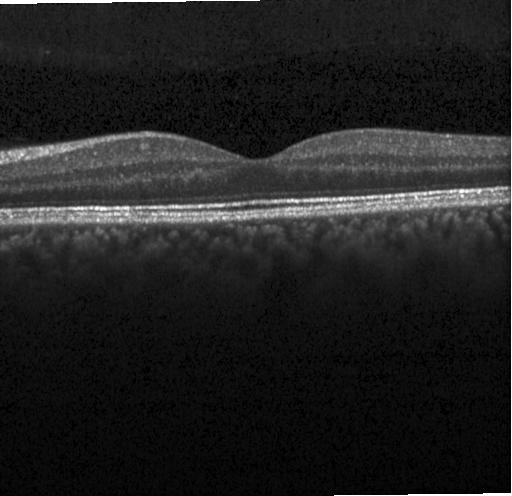

Macular OCT: no evidence of CNV, DME, or drusen.